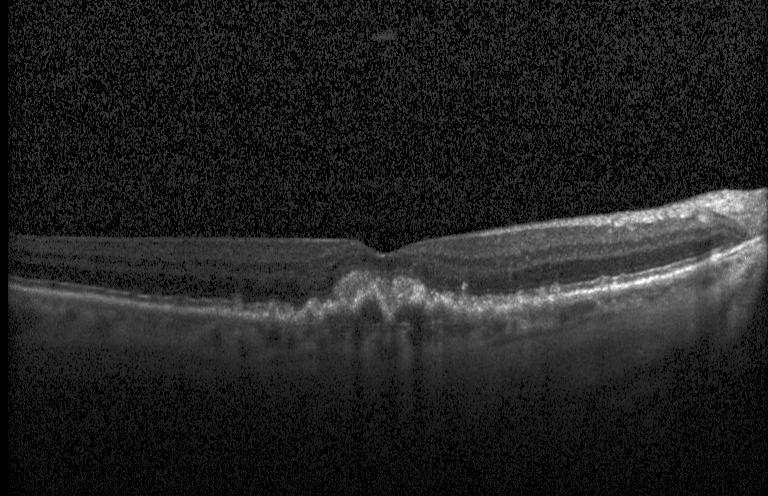 Spectral-domain OCT B-scan: CNV.